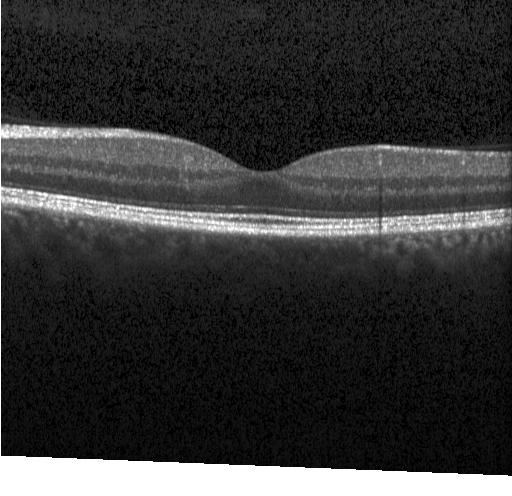

Finding: no choroidal neovascularization, diabetic macular edema, or drusen.